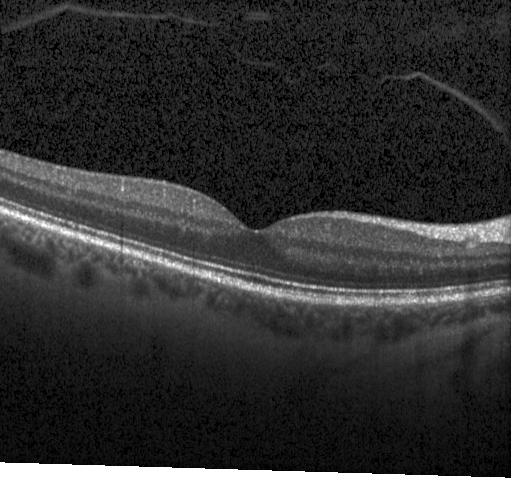

Acquired on a Heidelberg Spectralis · macular scan · optical coherence tomography scan.
No choroidal neovascularization, diabetic macular edema, or drusen.